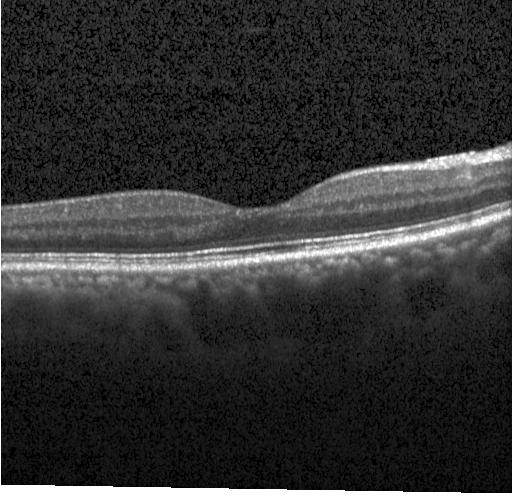

Instrument: Heidelberg Spectralis, through the macula, spectral-domain optical coherence tomography, optical coherence tomography scan.
Impression: no choroidal neovascularization, no diabetic macular edema, and no drusen.